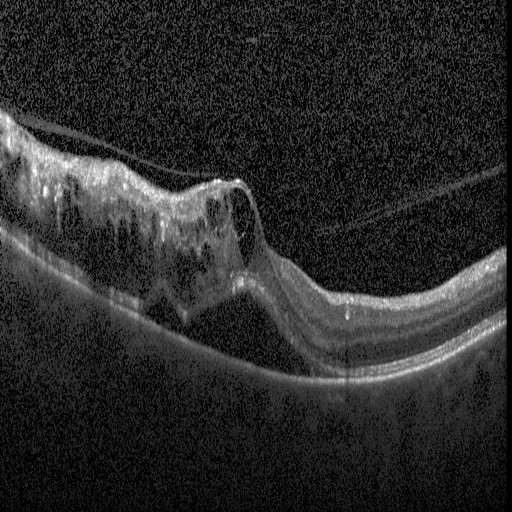
OCT B-scan.
Macular OCT: diabetic macular edema.